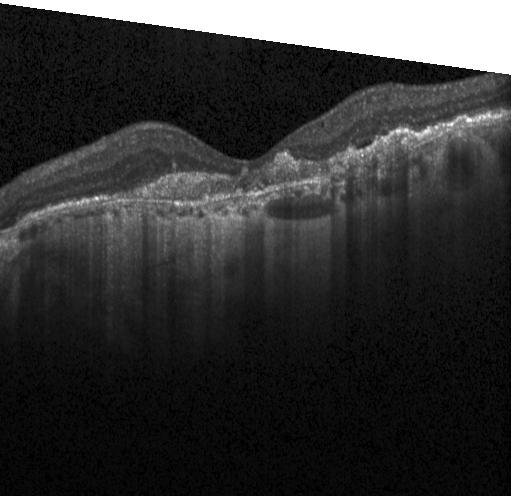
SD-OCT, Heidelberg Spectralis, retinal OCT cross-section, through the macula — Finding: a choroidal neovascular membrane.